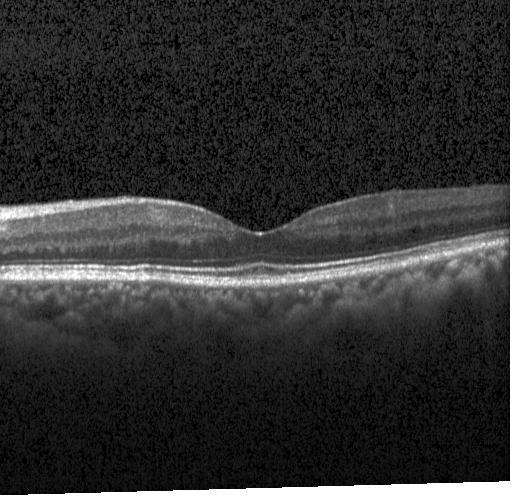

Retinal OCT B-scan; centered on the fovea; Heidelberg Spectralis — Dx: no evidence of choroidal neovascularization, diabetic macular edema, or drusen.